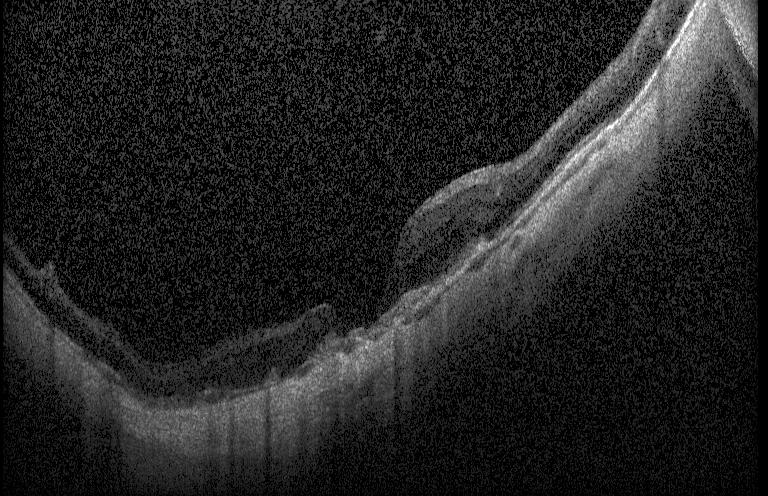 Retinal OCT cross-section showing a choroidal neovascular membrane.